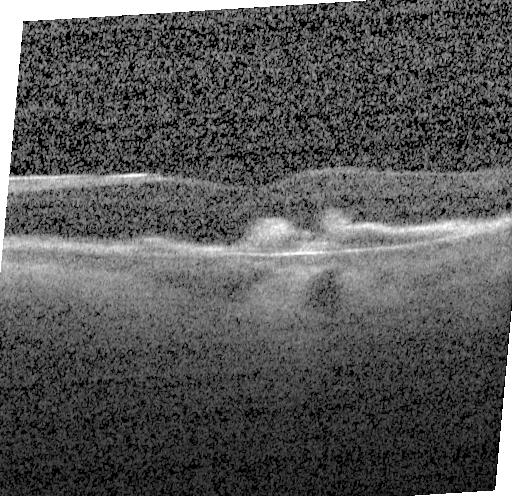

Spectral-domain OCT B-scan: a choroidal neovascular membrane.